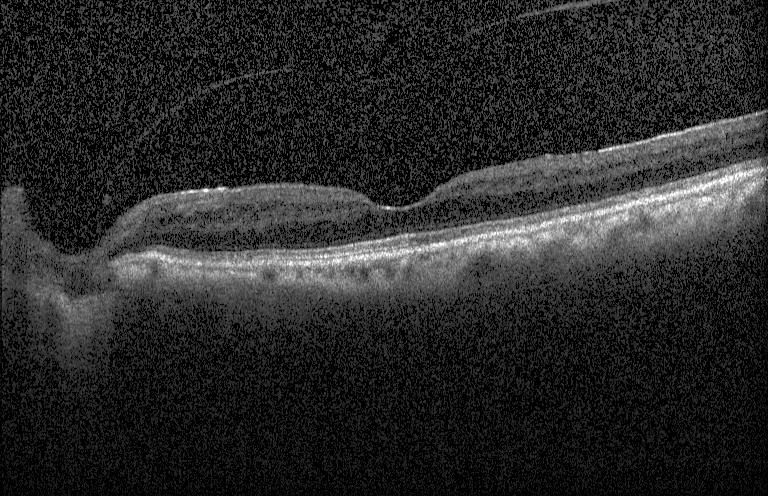
Through the macula; SD-OCT; acquired on a Heidelberg Spectralis; OCT line scan.
Impression: no evidence of CNV, DME, or drusen.